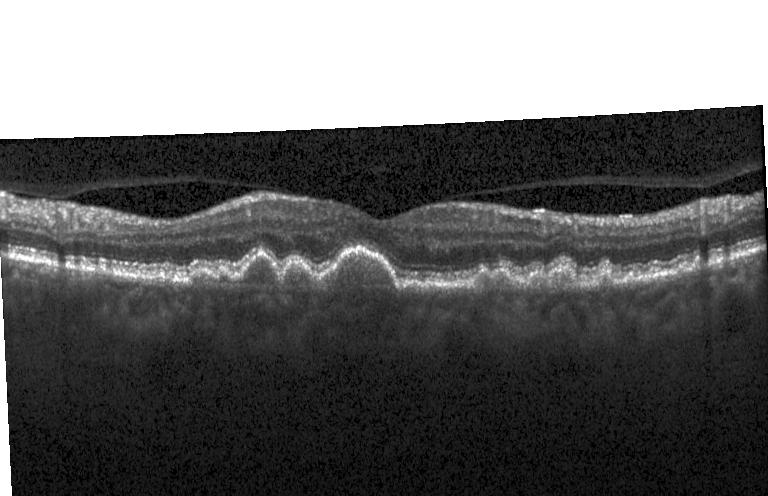
Finding: multiple drusen.